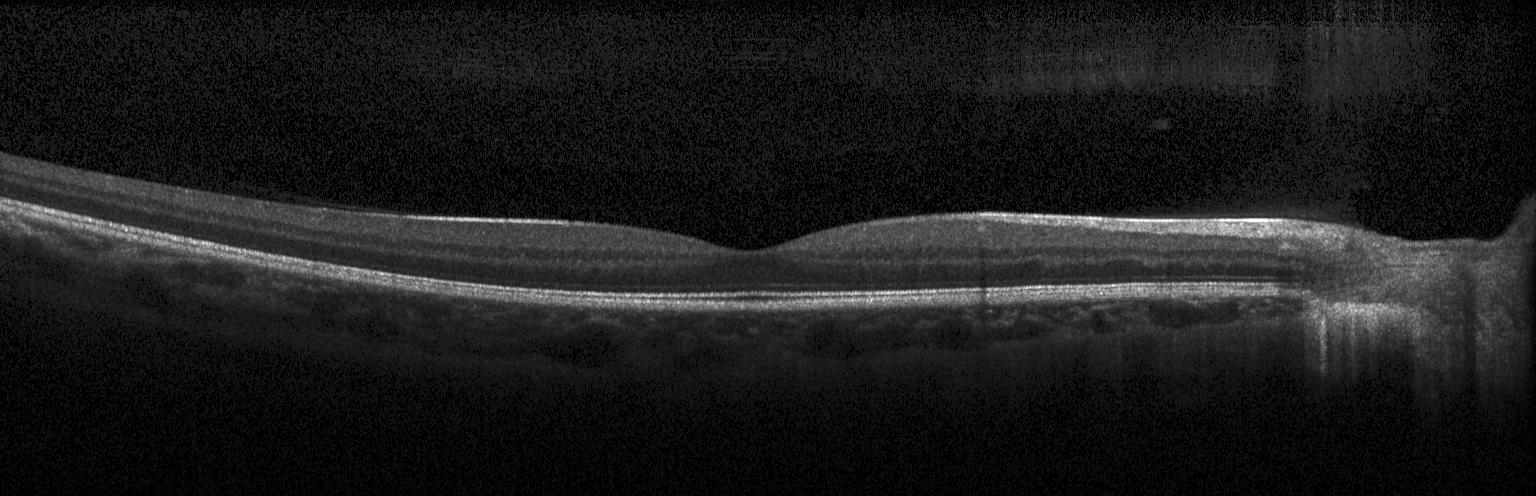

The scan shows no evidence of choroidal neovascularization, diabetic macular edema, or drusen.